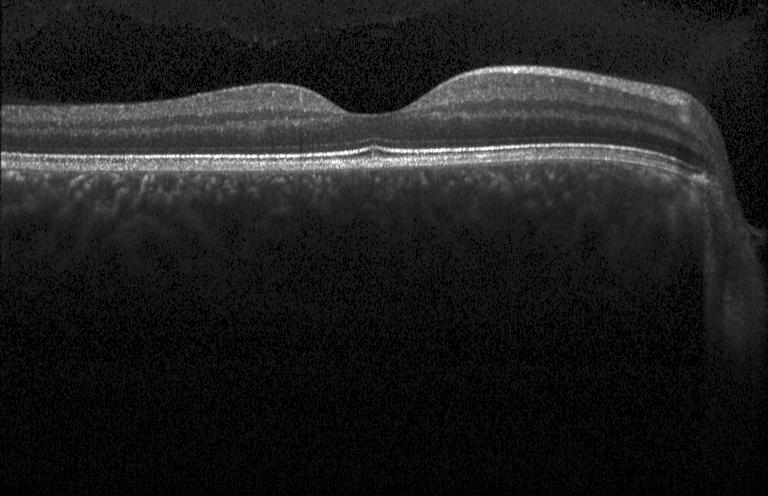 The scan shows no evidence of CNV, DME, or drusen.